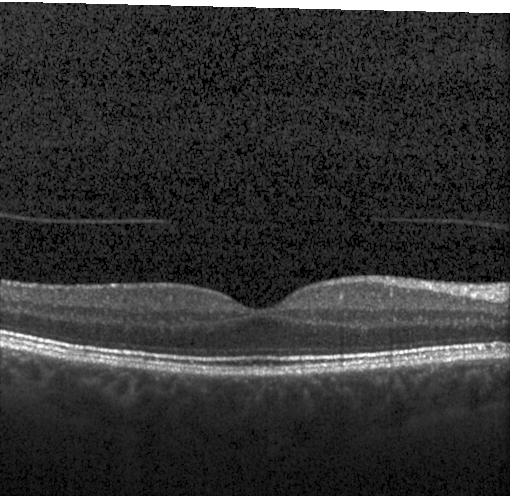

Centered on the fovea · OCT B-scan · SD-OCT · instrument: Heidelberg Spectralis.
Dx: neither CNV, DME, nor drusen.